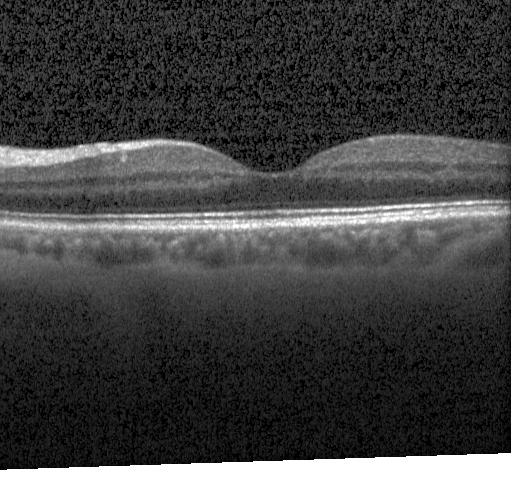
Macular OCT demonstrating neither choroidal neovascularization, diabetic macular edema, nor drusen.